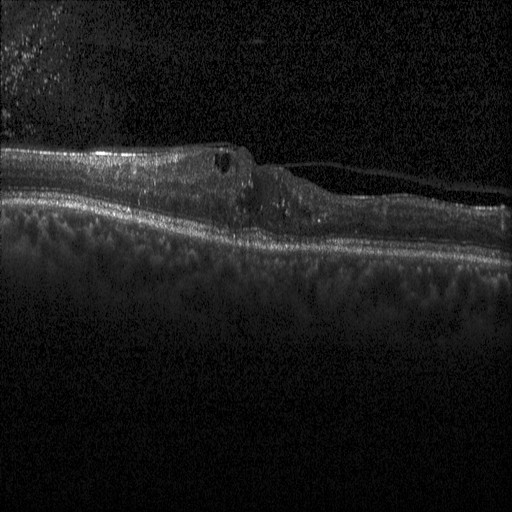 Retinal OCT B-scan · Heidelberg Spectralis OCT system.
Diagnosis: diabetic macular edema (DME).